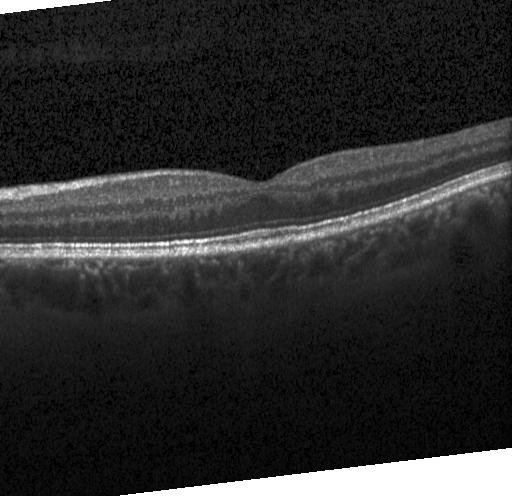
OCT B-scan, fovea-centered, acquired on a Heidelberg Spectralis. Finding: neither choroidal neovascularization, diabetic macular edema, nor drusen.